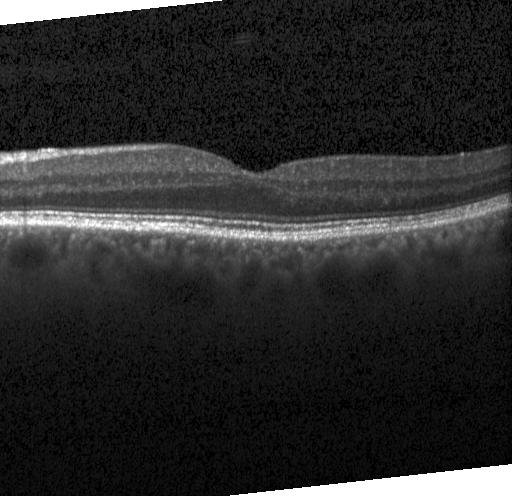

Optical coherence tomography B-scan.
This B-scan demonstrates no evidence of choroidal neovascularization, diabetic macular edema, or drusen.